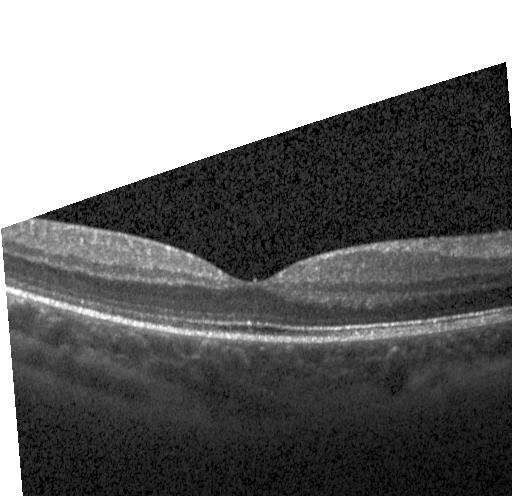 Spectral-domain OCT B-scan: neither choroidal neovascularization, diabetic macular edema, nor drusen.